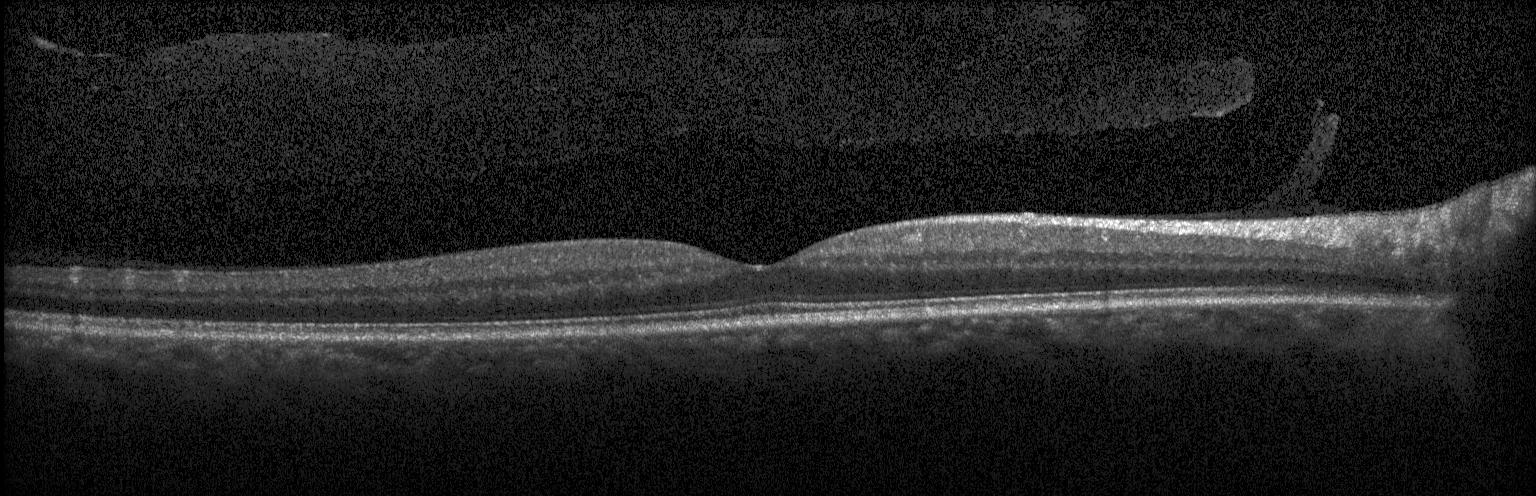

Impression: no evidence of CNV, DME, or drusen.